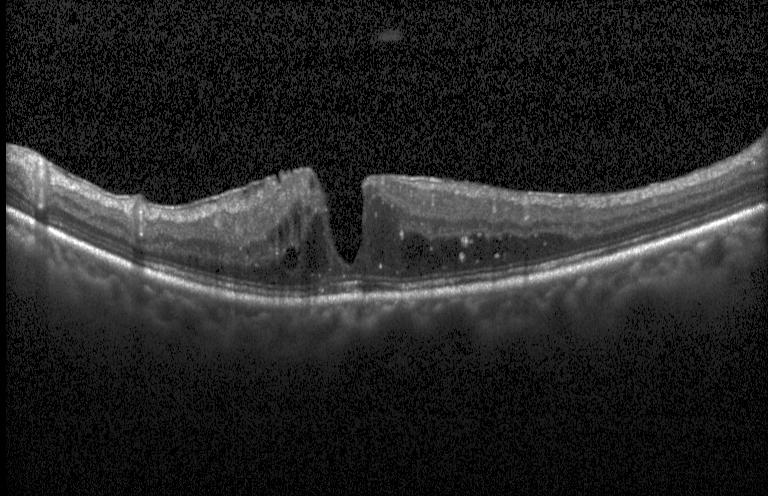

Heidelberg Spectralis OCT system; OCT B-scan; spectral-domain optical coherence tomography. OCT finding: DME.